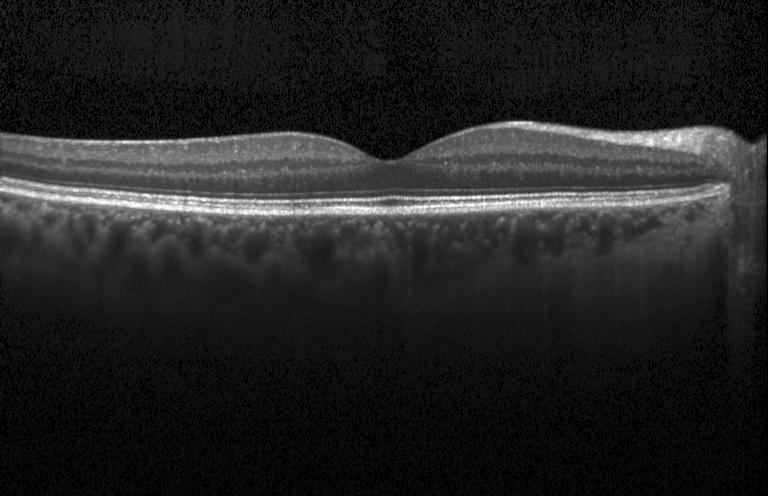 OCT line scan. Finding: no choroidal neovascularization, no diabetic macular edema, and no drusen.